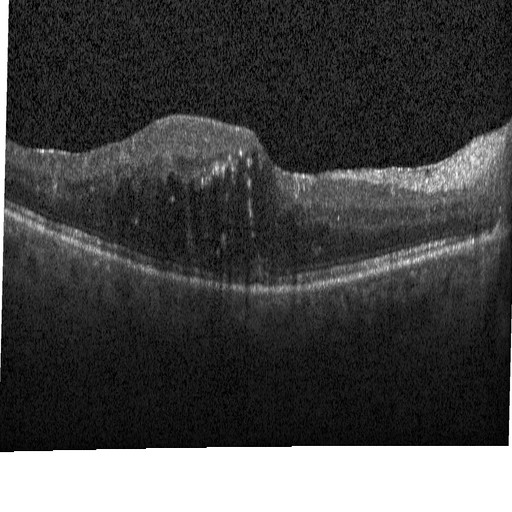
SD-OCT; acquired on a Heidelberg Spectralis; retinal OCT cross-section; through the macula. This B-scan demonstrates diabetic macular edema (DME).